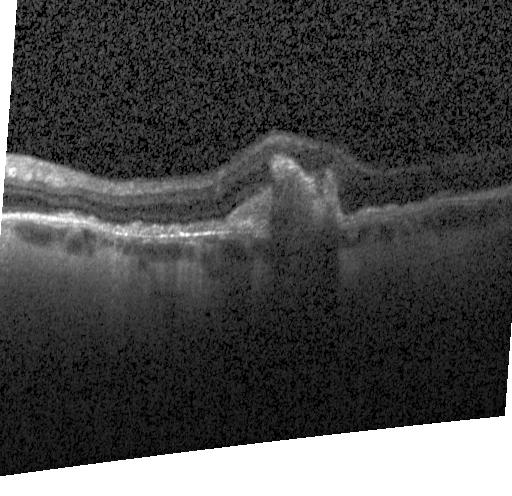 Optical coherence tomography scan — Diagnosis: choroidal neovascularization (CNV).